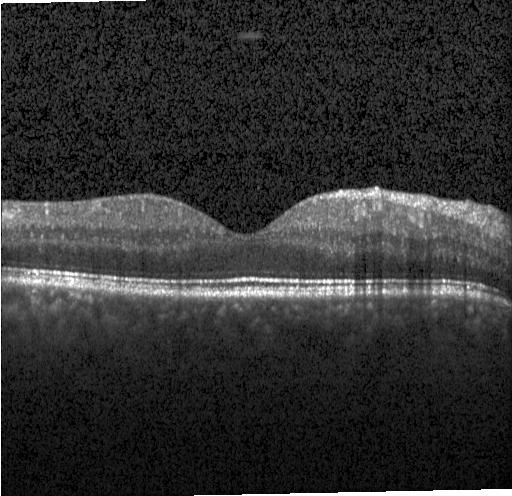 OCT line scan — No choroidal neovascularization, no diabetic macular edema, and no drusen.